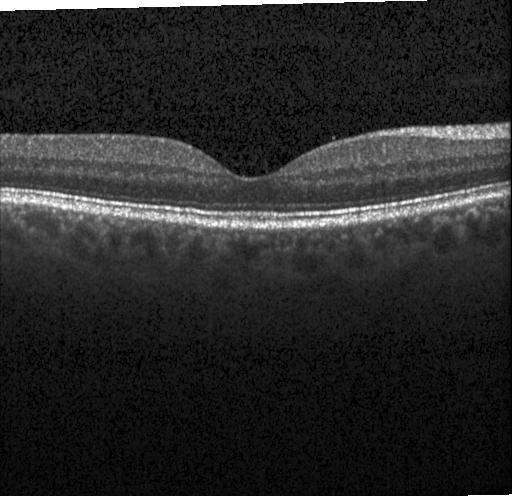 OCT B-scan · instrument: Heidelberg Spectralis. Finding: no choroidal neovascularization, diabetic macular edema, or drusen.